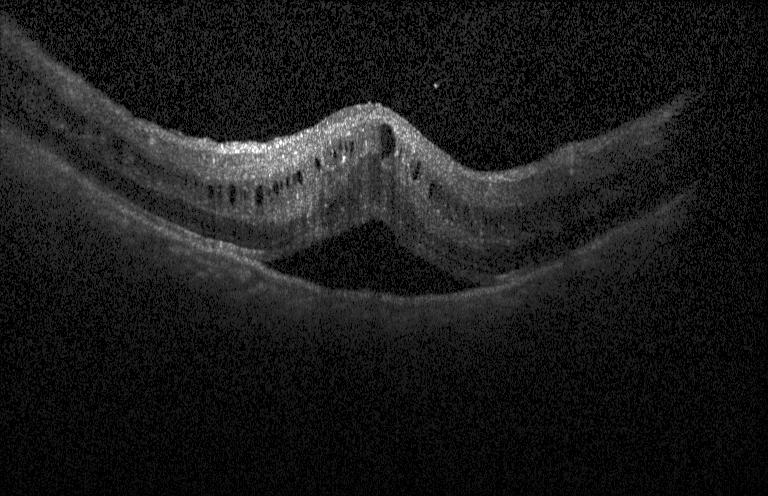

SD-OCT, retinal OCT cross-section
Finding: diabetic macular edema (DME).